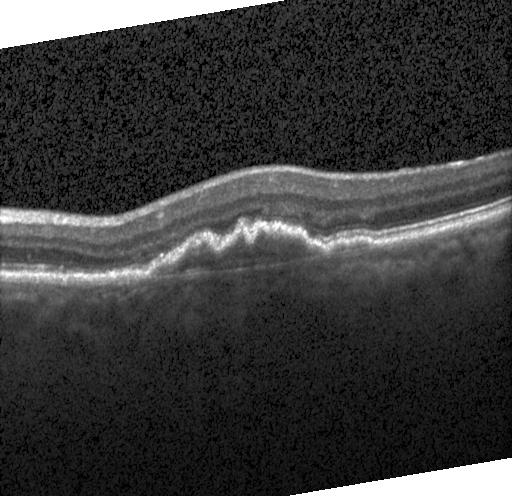
Choroidal neovascularization.